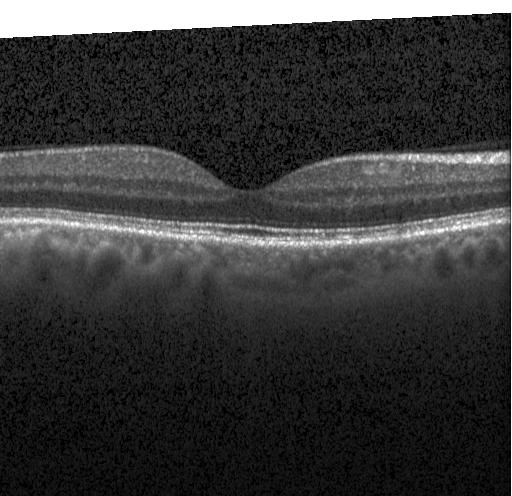 Dx: no CNV, DME, or drusen.